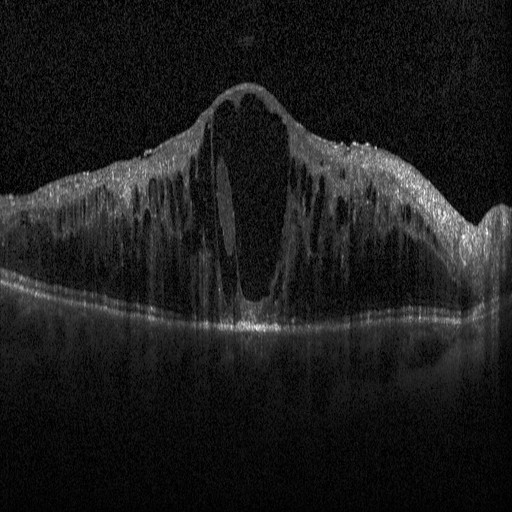
Dx: diabetic macular edema.